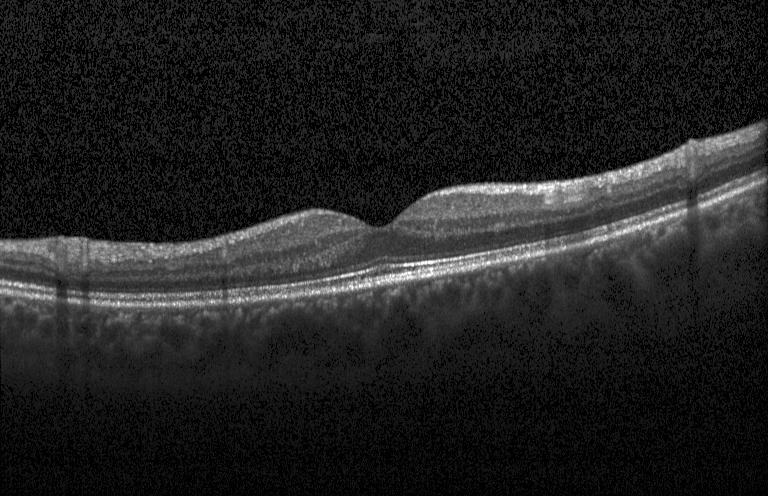

Retinal OCT B-scan. Heidelberg Spectralis. Centered on the fovea
Finding: no evidence of choroidal neovascularization, diabetic macular edema, or drusen.